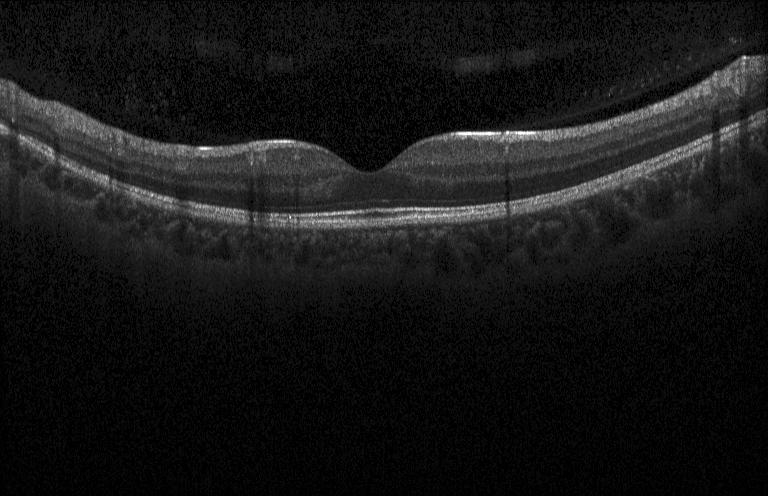 Macular OCT: no CNV, no DME, and no drusen.